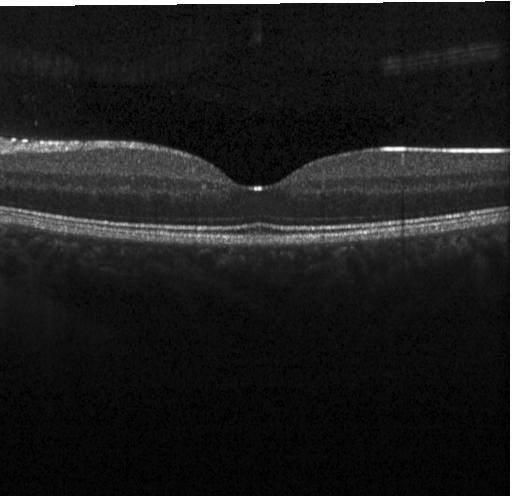 Heidelberg Spectralis OCT system, fovea-centered, SD-OCT, optical coherence tomography B-scan — Assessment: neither CNV, DME, nor drusen.